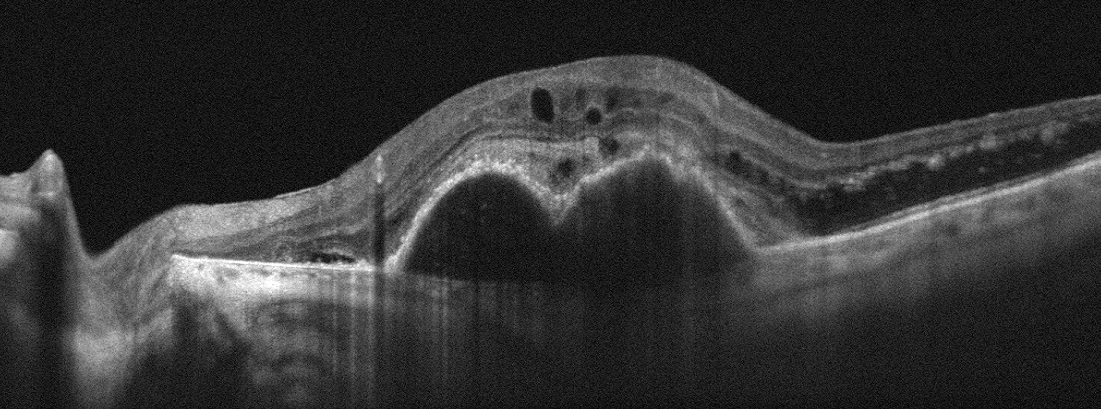

Macular OCT: AMD.